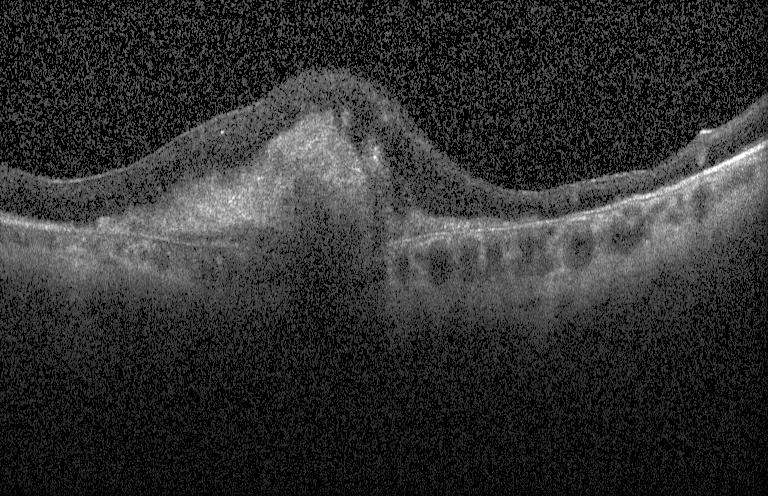

Retinal OCT cross-section; acquired on a Heidelberg Spectralis — OCT finding: choroidal neovascularization (CNV).